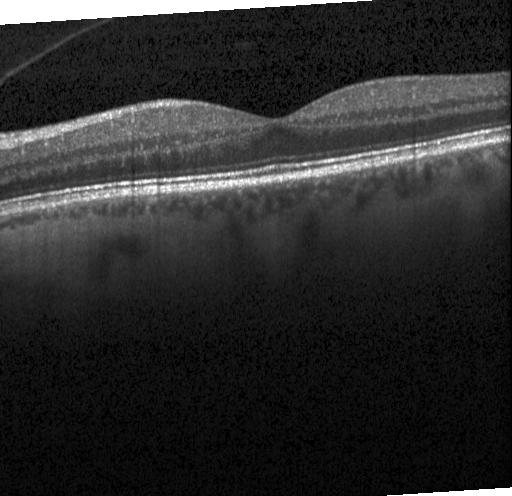

Optical coherence tomography scan; fovea-centered; Heidelberg Spectralis OCT system; spectral-domain optical coherence tomography. Finding: neither choroidal neovascularization, diabetic macular edema, nor drusen.